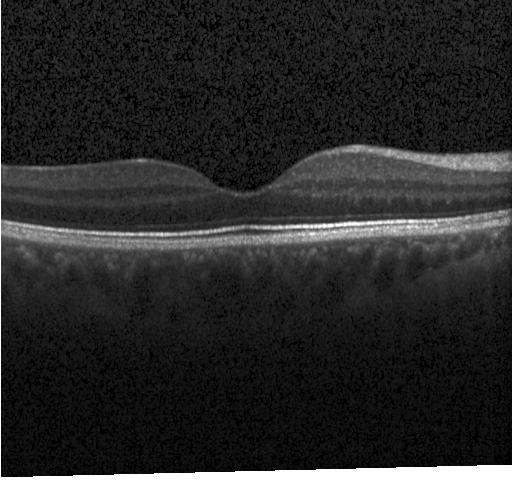 Impression: no choroidal neovascularization, no diabetic macular edema, and no drusen.